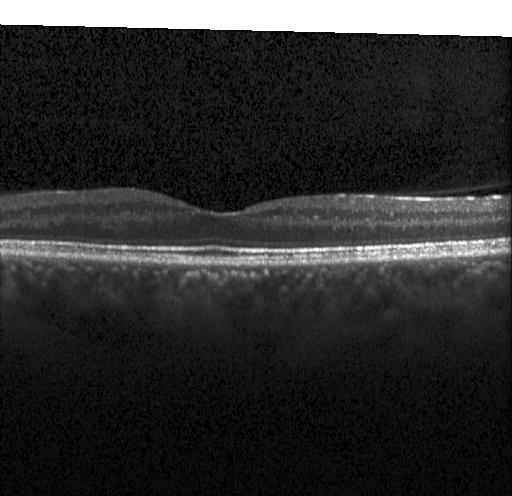

OCT B-scan showing no evidence of choroidal neovascularization, diabetic macular edema, or drusen.